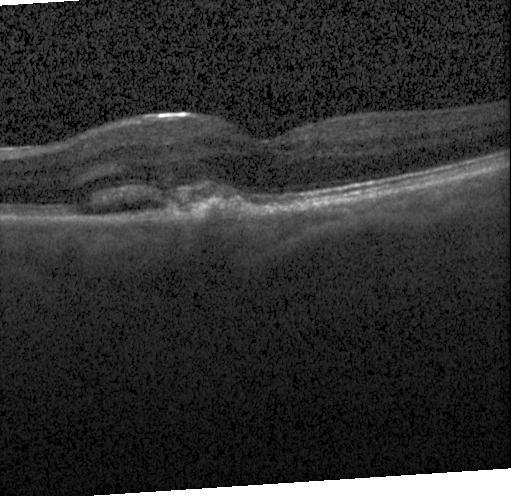

Diagnosis: a choroidal neovascular membrane.